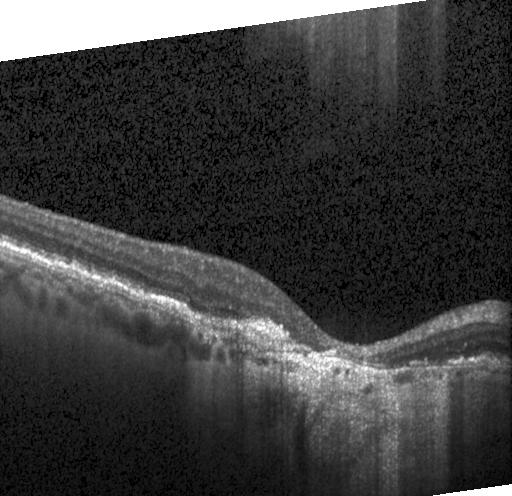
Retinal OCT B-scan — Assessment: a choroidal neovascular membrane.